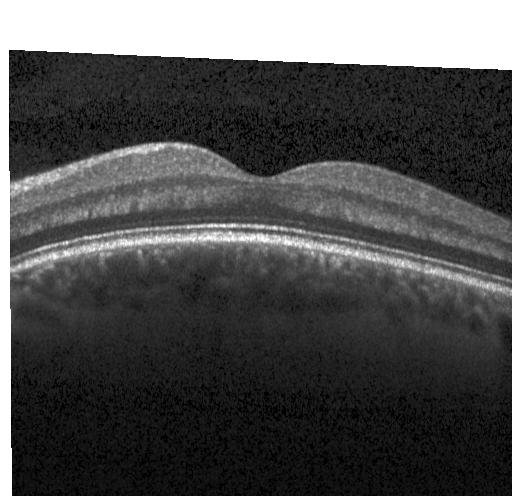 Heidelberg Spectralis · optical coherence tomography scan — OCT finding: neither choroidal neovascularization, diabetic macular edema, nor drusen.